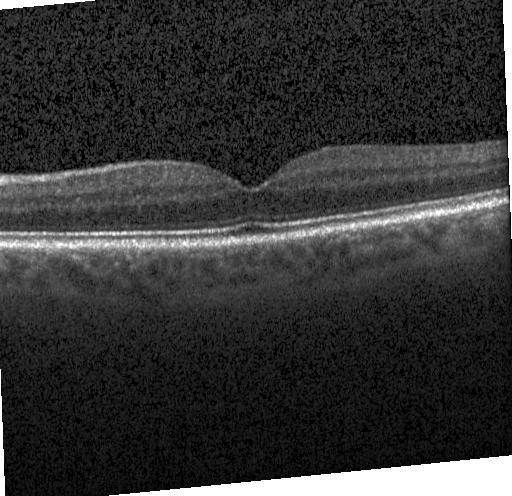
Retinal OCT B-scan; acquired on a Heidelberg Spectralis; centered on the fovea; spectral-domain optical coherence tomography. Finding: no choroidal neovascularization, no diabetic macular edema, and no drusen.